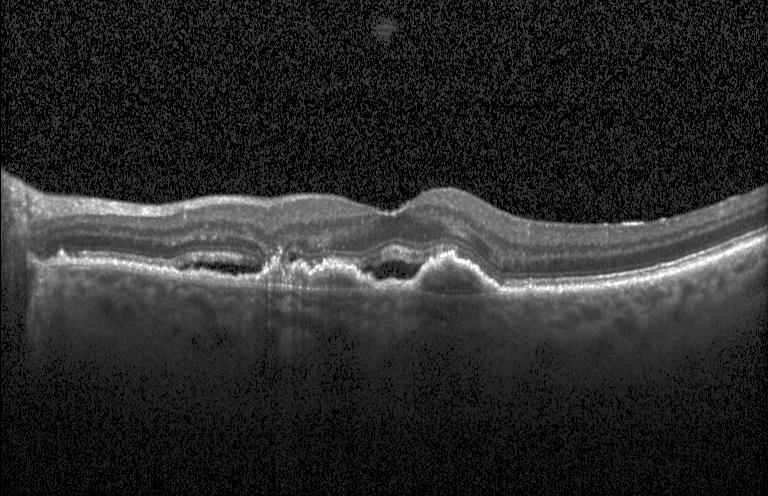 Impression: a choroidal neovascular membrane.